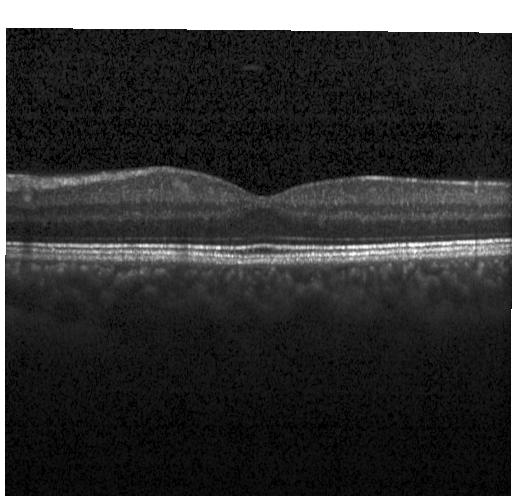 Finding: no evidence of choroidal neovascularization, diabetic macular edema, or drusen.